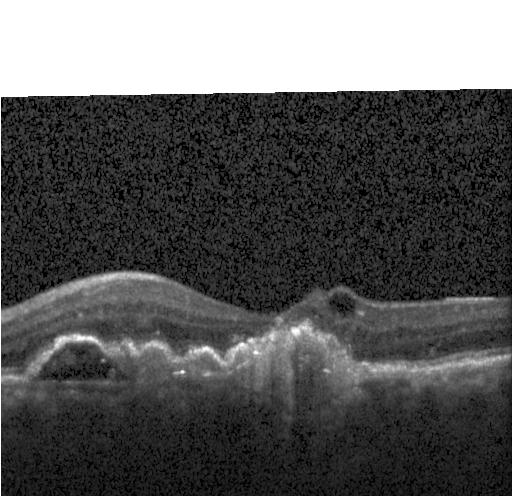 OCT B-scan
Impression: choroidal neovascularization (CNV).